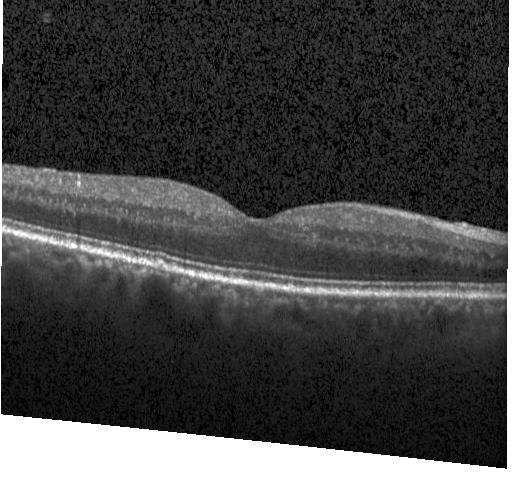

Optical coherence tomography B-scan — Neither choroidal neovascularization, diabetic macular edema, nor drusen.